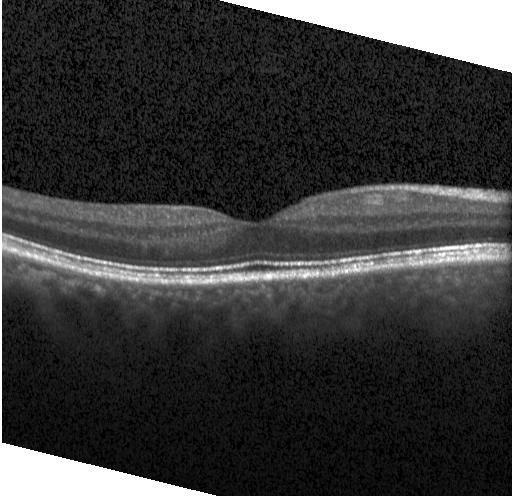

Finding: no choroidal neovascularization, diabetic macular edema, or drusen.